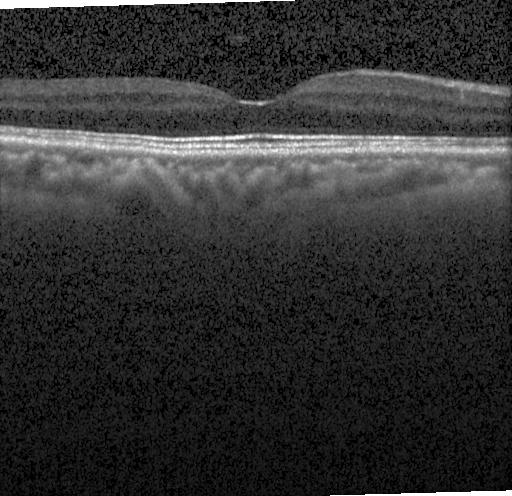
Macular OCT: no choroidal neovascularization, diabetic macular edema, or drusen.